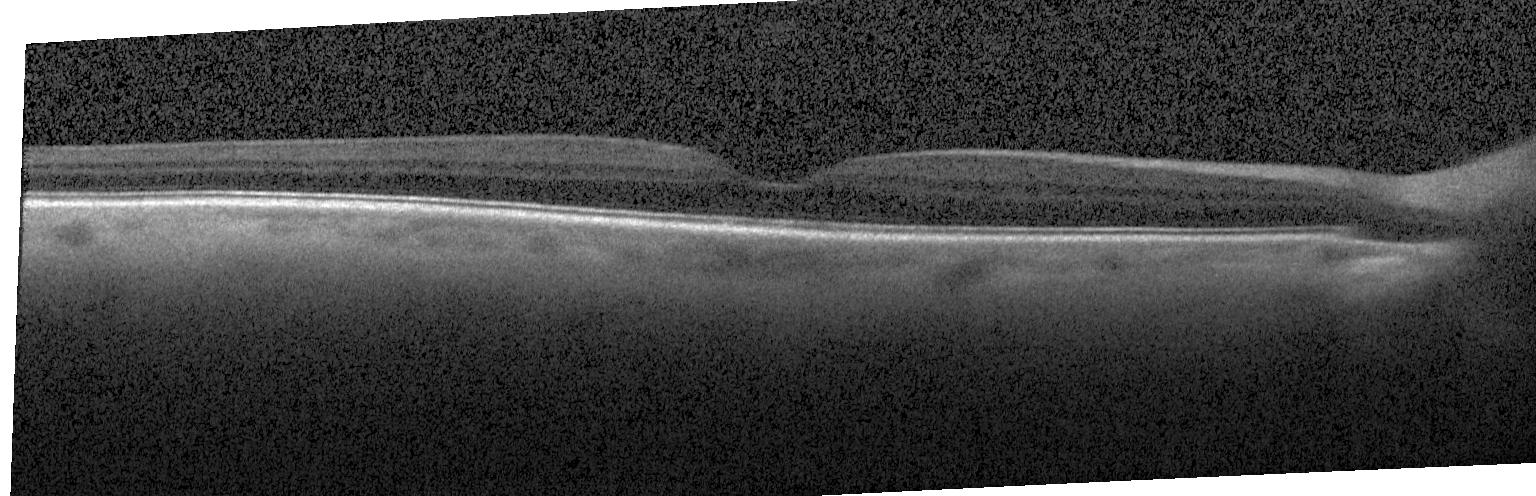

Diagnosis: no CNV, DME, or drusen.